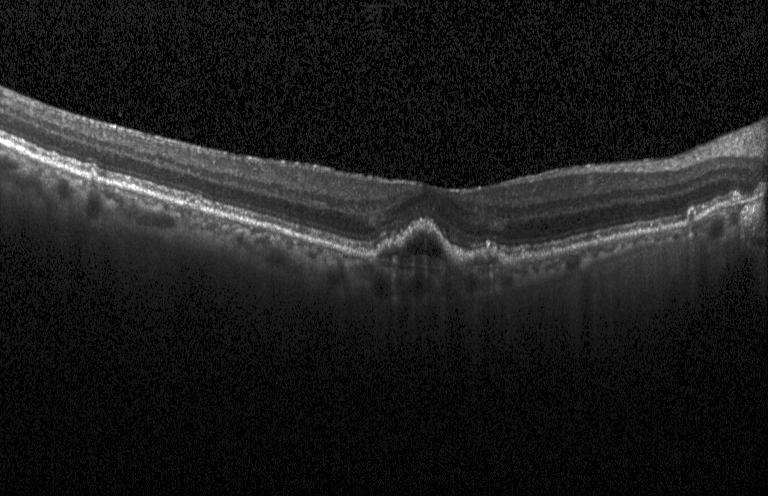 Retinal OCT cross-section; SD-OCT
A choroidal neovascular membrane.